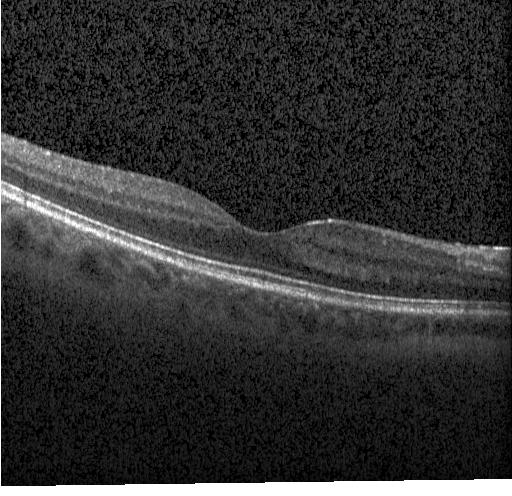 Finding: no evidence of choroidal neovascularization, diabetic macular edema, or drusen.